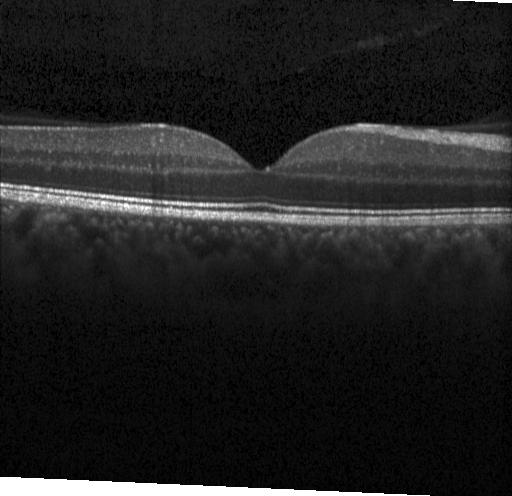 Through the macula, Heidelberg Spectralis, retinal OCT cross-section, spectral-domain optical coherence tomography
Impression: neither choroidal neovascularization, diabetic macular edema, nor drusen.